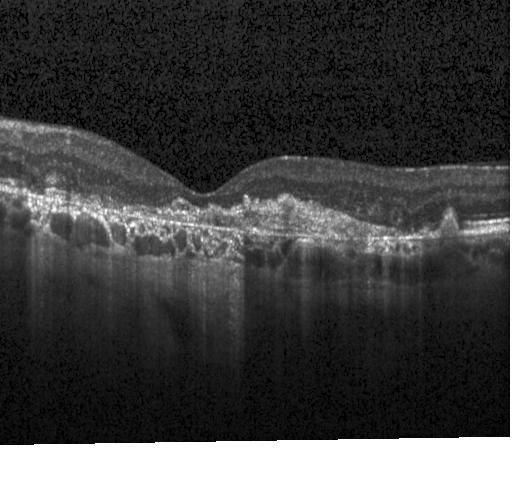
This B-scan demonstrates a choroidal neovascular membrane.